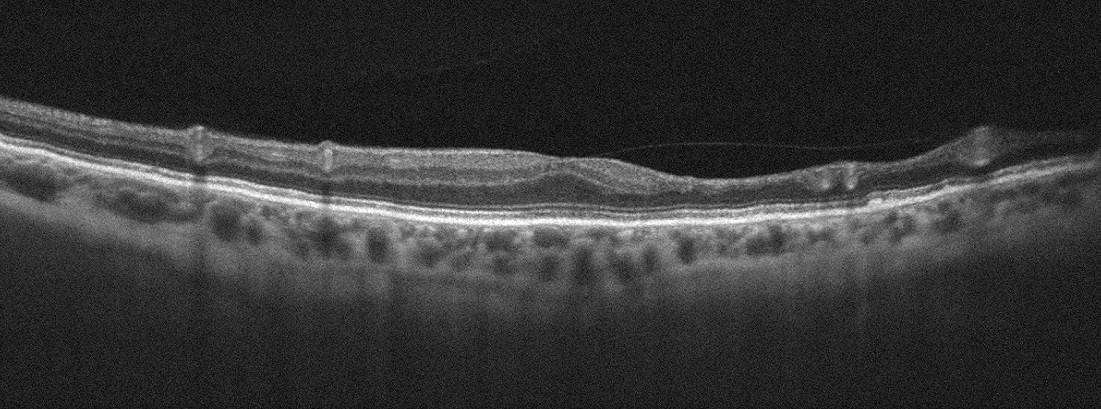 Retinal OCT cross-section; acquired on an Optovue Avanti RTVue XR.
This B-scan demonstrates RVO.